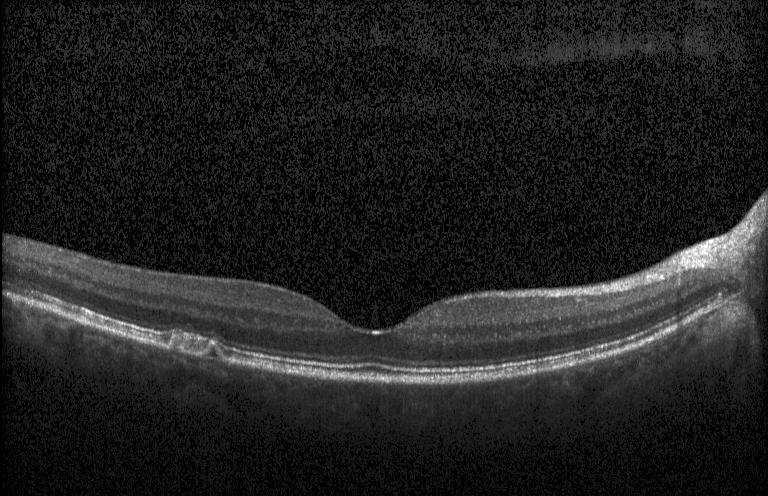
OCT B-scan. Heidelberg Spectralis. Horizontal scan through the fovea. Spectral-domain OCT. Impression: no choroidal neovascularization, no diabetic macular edema, and no drusen.